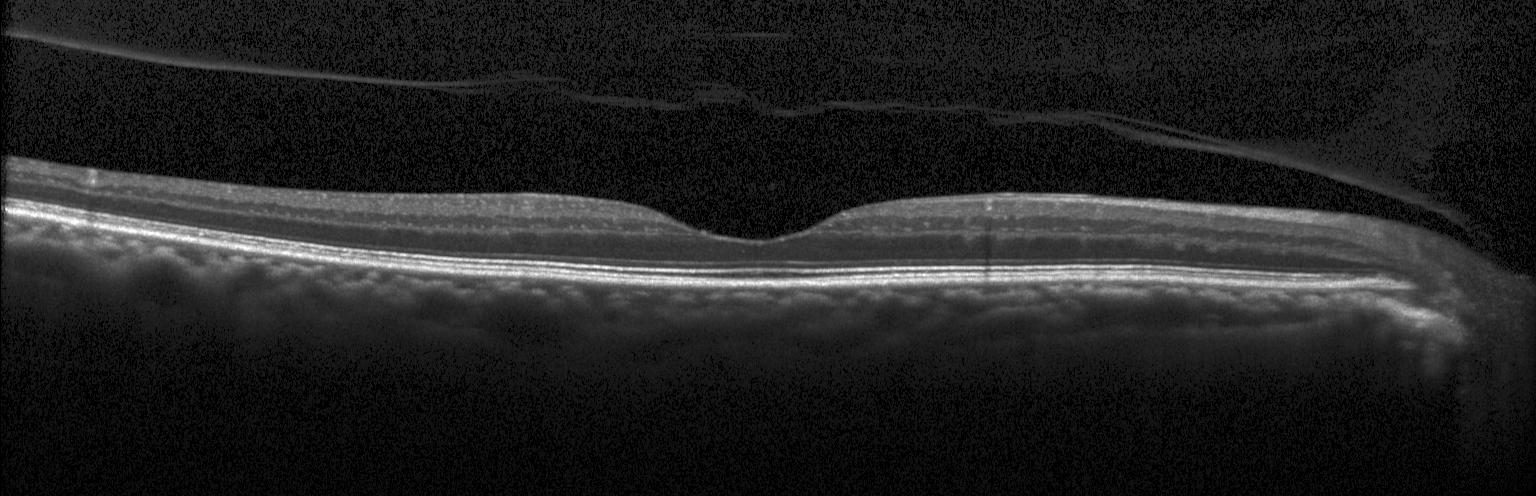

Retinal OCT B-scan · SD-OCT — This B-scan demonstrates no choroidal neovascularization, no diabetic macular edema, and no drusen.